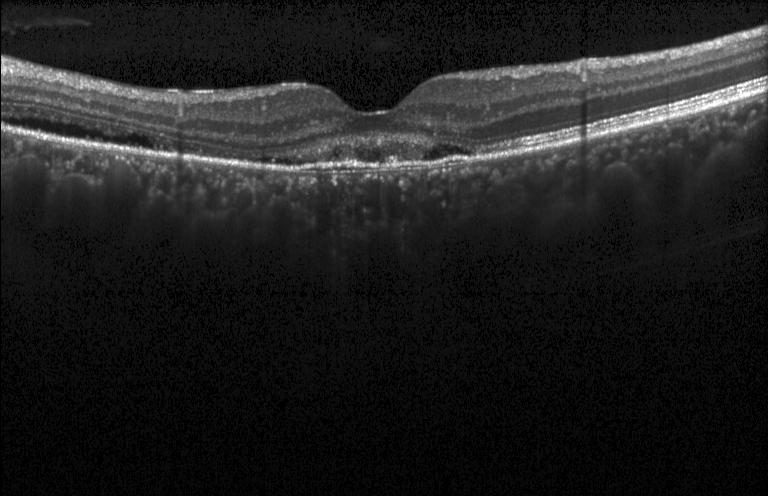
Macular OCT: CNV.